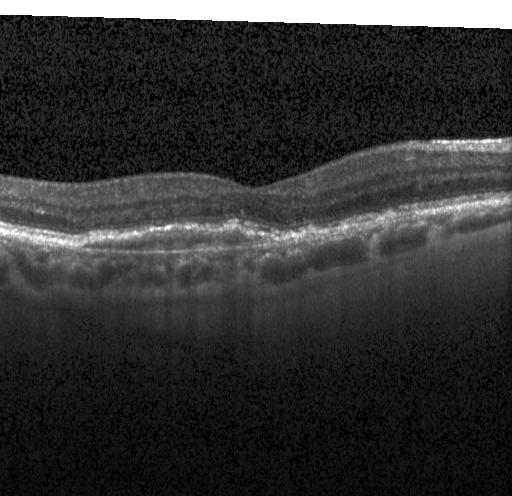

Diagnosis: choroidal neovascularization (CNV).